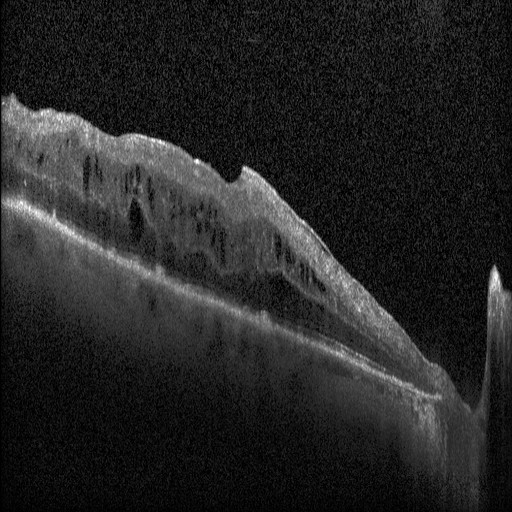
Impression: DME.